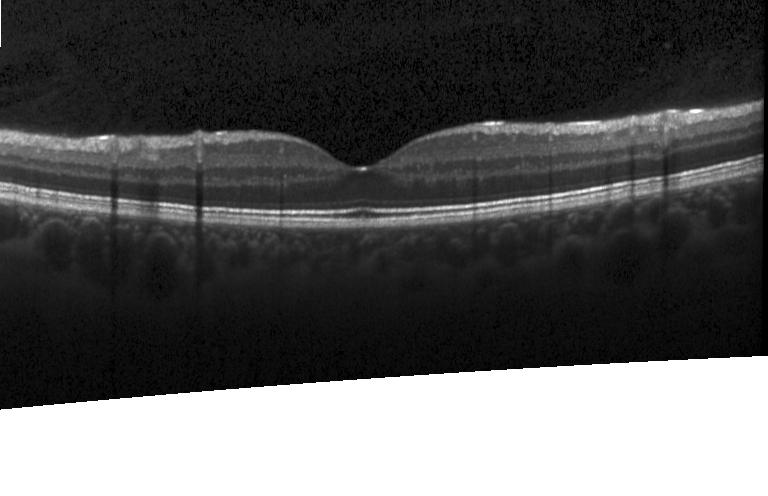
OCT B-scan · fovea-centered · acquired on a Heidelberg Spectralis · spectral-domain OCT. Impression: neither choroidal neovascularization, diabetic macular edema, nor drusen.